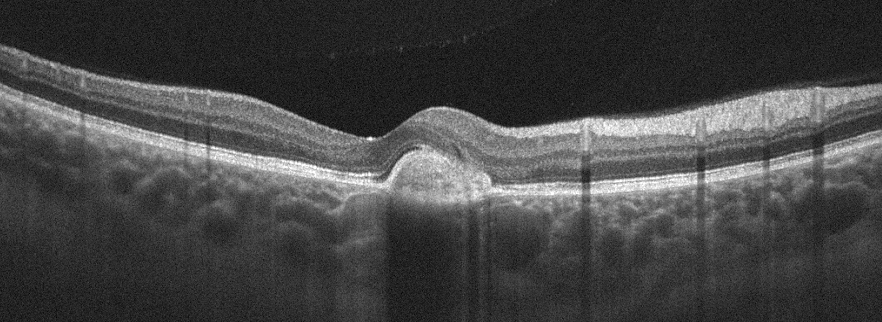
Optovue Avanti RTVue XR, OCT line scan, macular scan, OS.
The scan shows age-related macular degeneration (AMD).